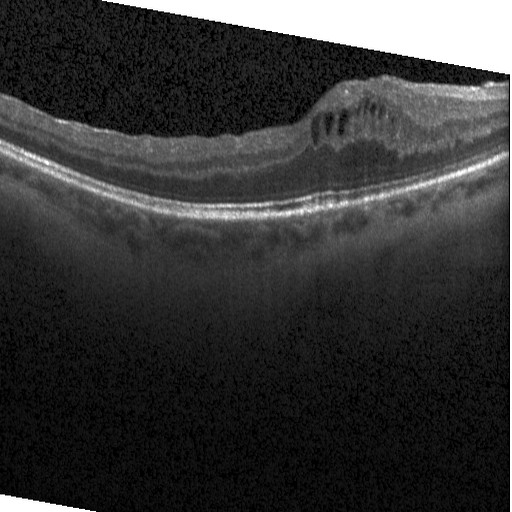

Heidelberg Spectralis · OCT B-scan · spectral-domain OCT
The scan shows diabetic macular edema.